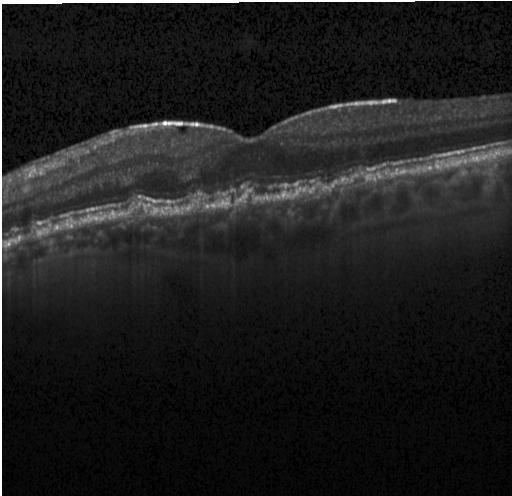

Finding: sub-RPE drusenoid deposits.